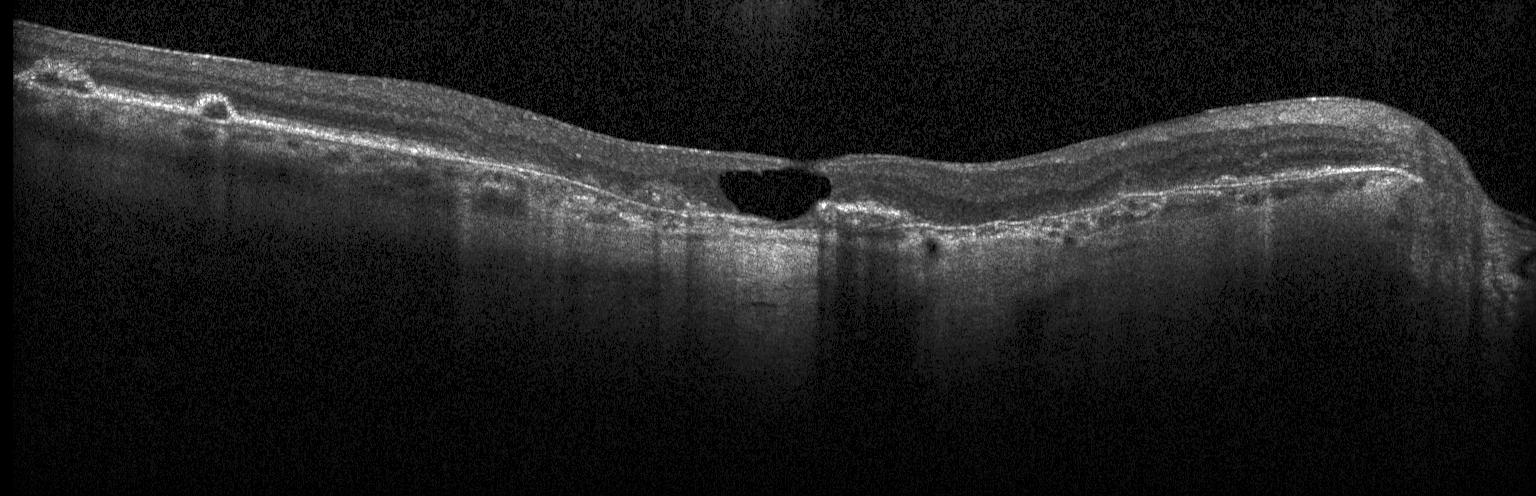

Heidelberg Spectralis OCT system · retinal OCT cross-section
Finding: choroidal neovascularization.